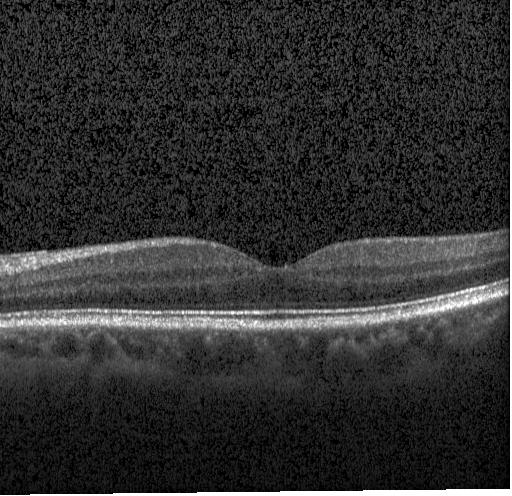

Retinal OCT cross-section; SD-OCT; Heidelberg Spectralis OCT system; fovea-centered — Impression: no choroidal neovascularization, no diabetic macular edema, and no drusen.